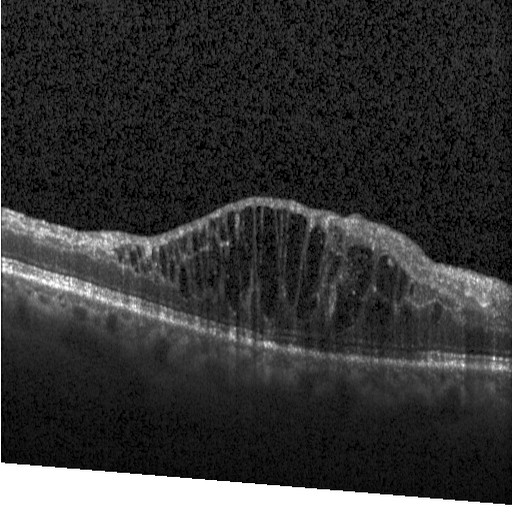
Assessment: diabetic macular edema.